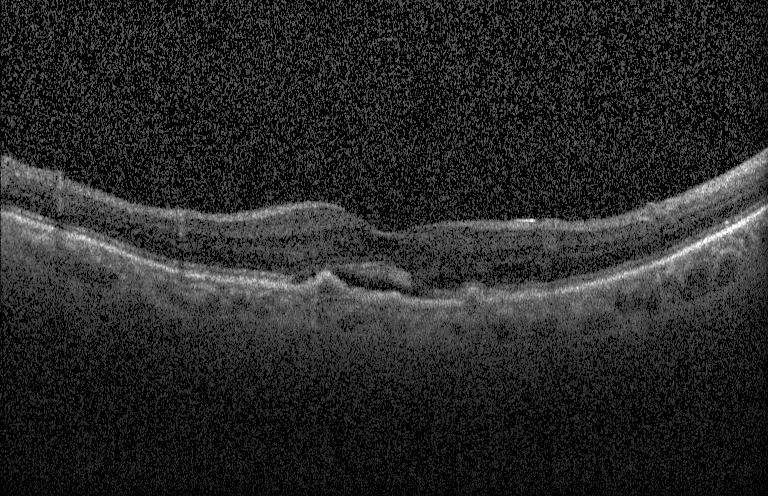
Macular OCT: a choroidal neovascular membrane.